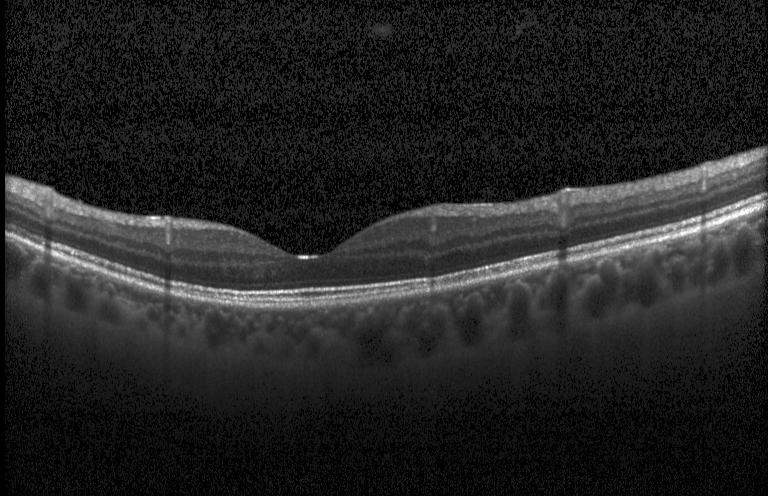
SD-OCT · OCT line scan.
This B-scan demonstrates no choroidal neovascularization, no diabetic macular edema, and no drusen.